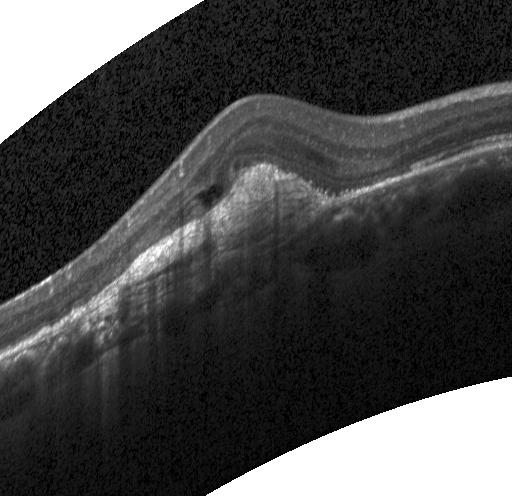
OCT line scan. OCT finding: choroidal neovascularization (CNV).